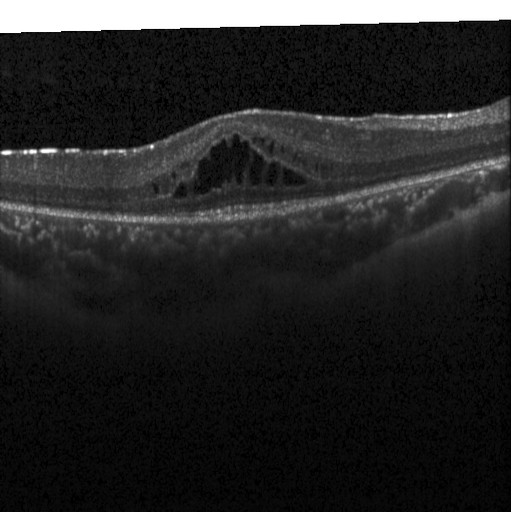 Macular OCT demonstrating DME.